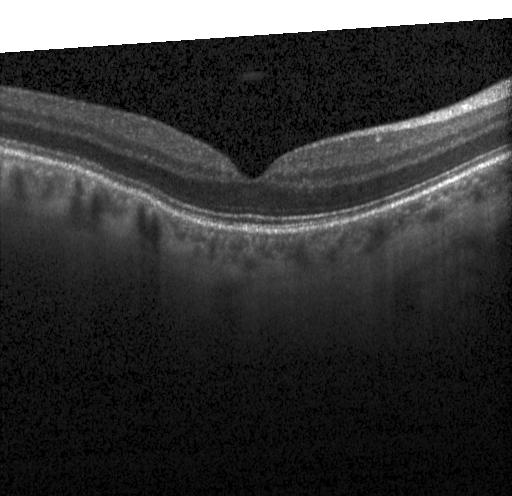

OCT line scan, spectral-domain optical coherence tomography, through the macula — Finding: no evidence of choroidal neovascularization, diabetic macular edema, or drusen.